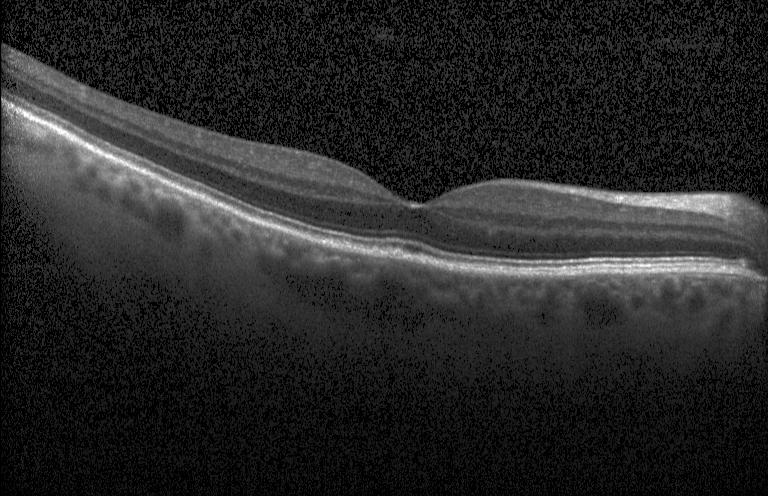

OCT B-scan, instrument: Heidelberg Spectralis
OCT finding: no evidence of choroidal neovascularization, diabetic macular edema, or drusen.